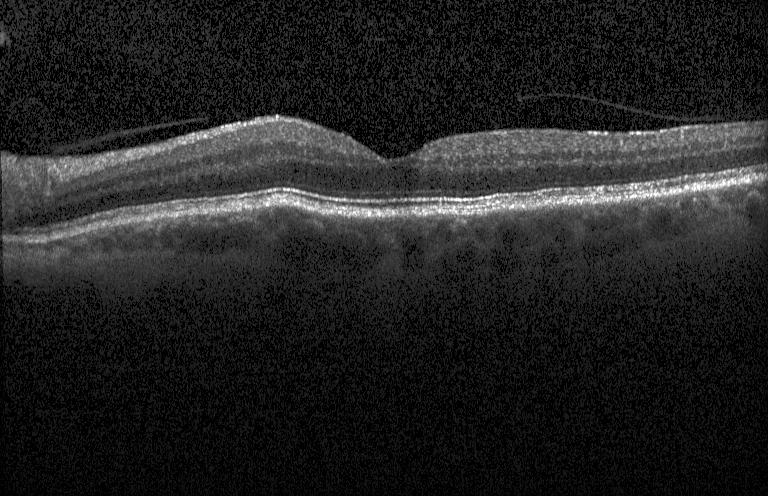
Retinal OCT cross-section · horizontal scan through the fovea. Macular OCT: neither CNV, DME, nor drusen.